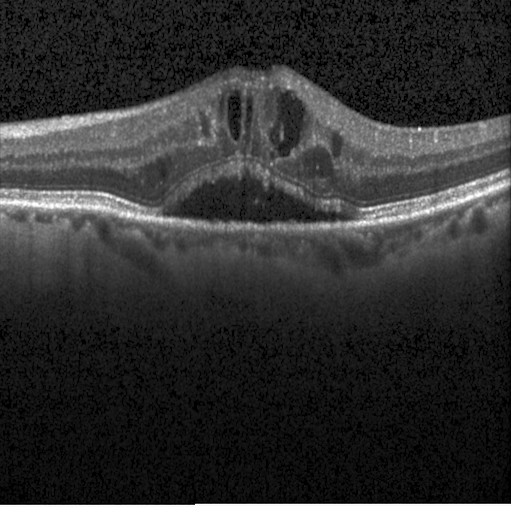 OCT B-scan
OCT finding: diabetic macular edema (DME).